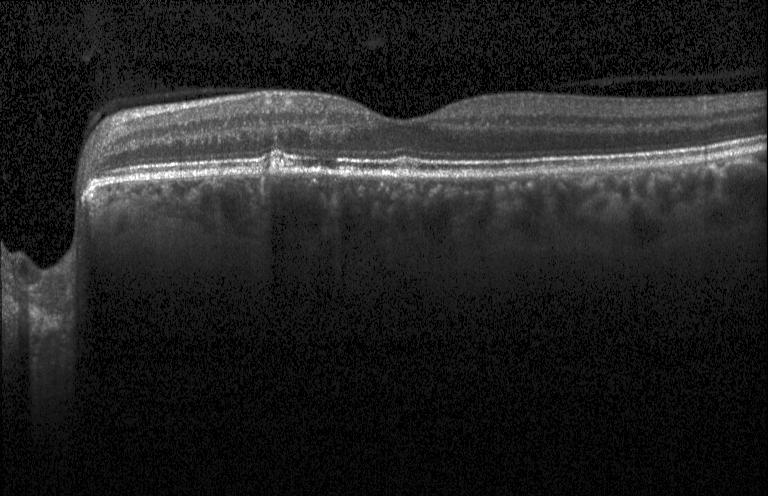
Spectral-domain OCT; Heidelberg Spectralis OCT system; macular scan; retinal OCT cross-section. Diagnosis: multiple drusen.